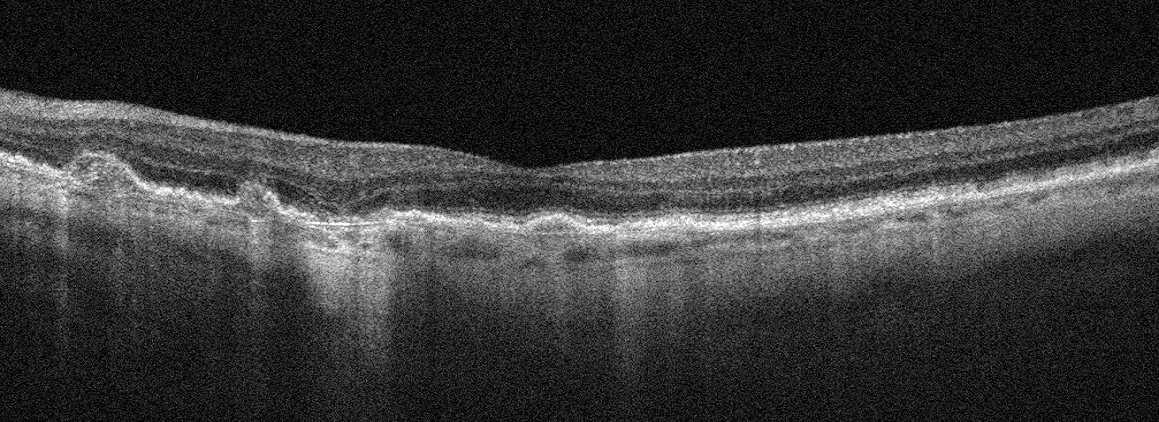

Left eye. Optical coherence tomography B-scan
Impression: AMD.